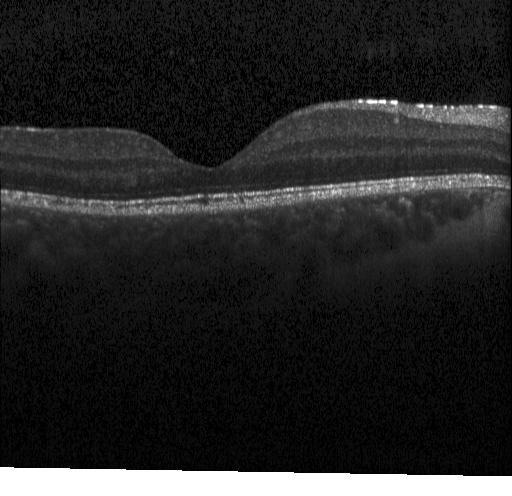 Optical coherence tomography scan — Finding: neither choroidal neovascularization, diabetic macular edema, nor drusen.